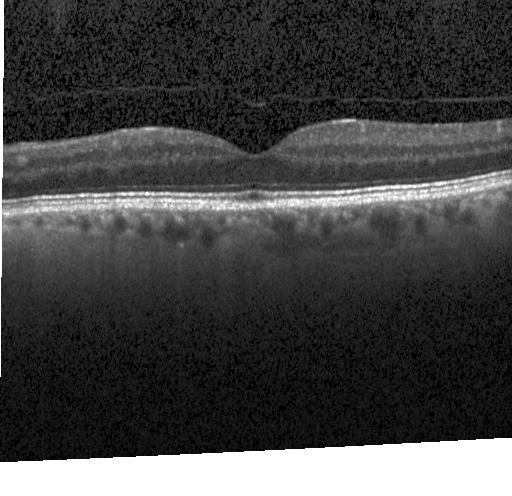 Retinal OCT cross-section; Heidelberg Spectralis OCT system; spectral-domain optical coherence tomography; centered on the fovea. Diagnosis: no choroidal neovascularization, diabetic macular edema, or drusen.